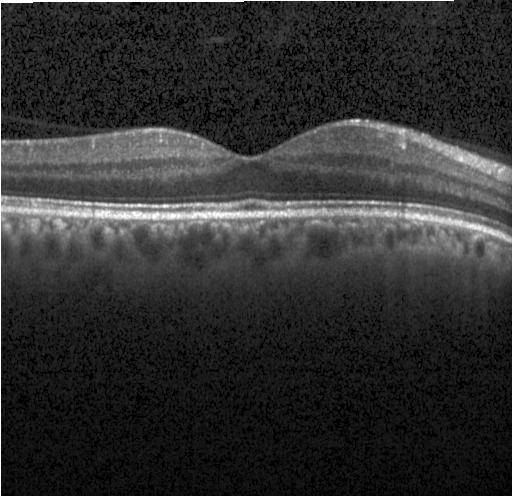

Finding: no choroidal neovascularization, no diabetic macular edema, and no drusen.